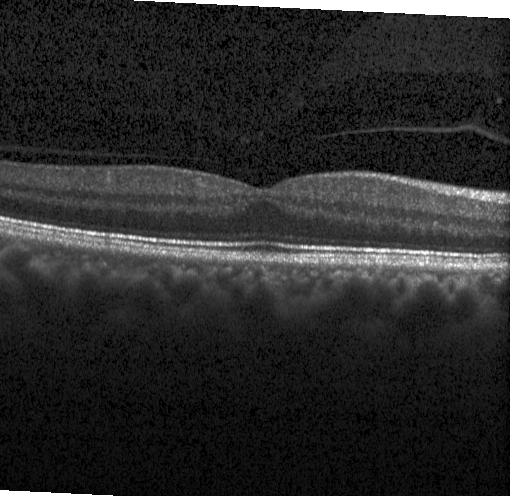
OCT line scan
Dx: neither choroidal neovascularization, diabetic macular edema, nor drusen.